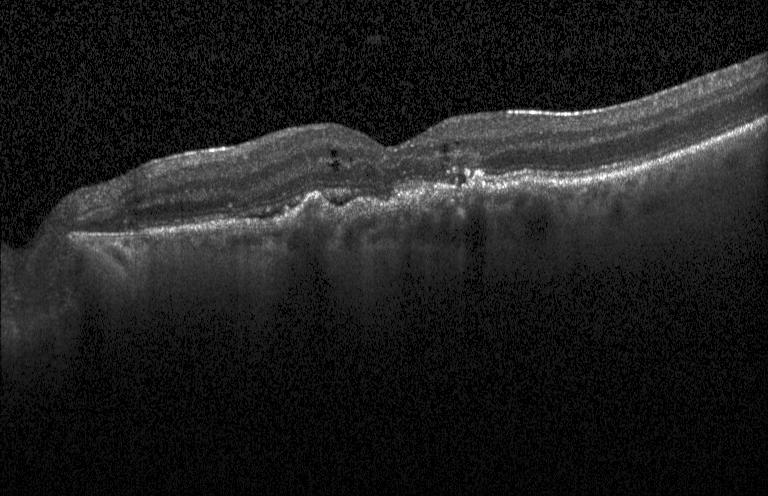
OCT B-scan showing choroidal neovascularization.